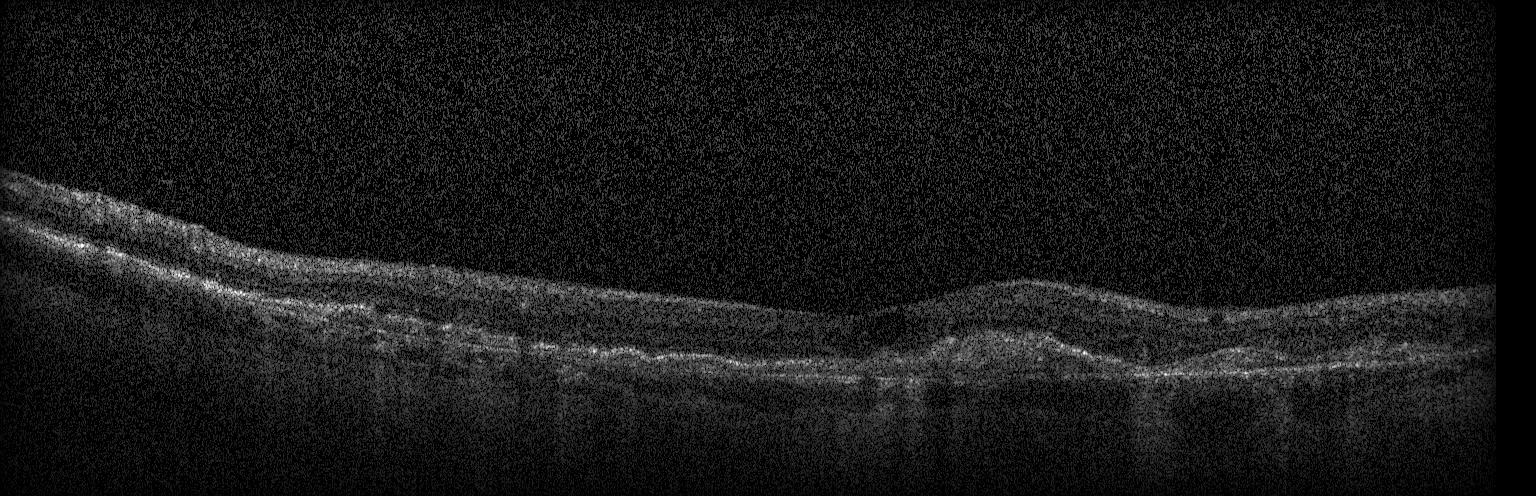
OCT B-scan. Diagnosis: CNV.